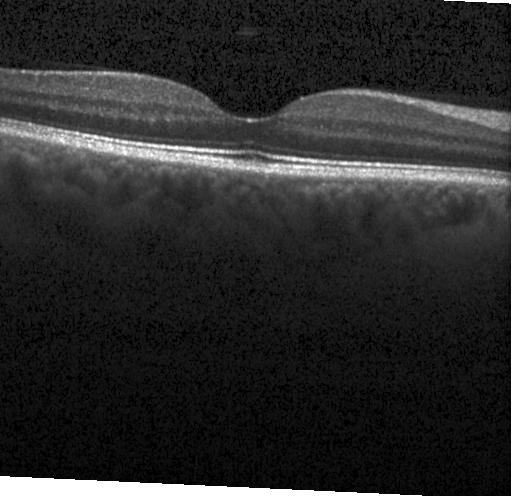
The scan shows no evidence of choroidal neovascularization, diabetic macular edema, or drusen.